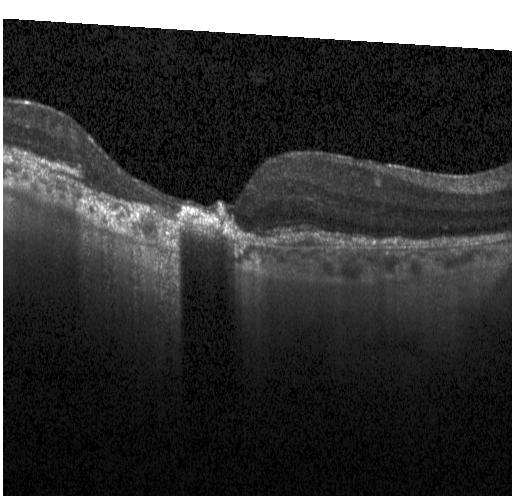
Optical coherence tomography B-scan. Assessment: CNV.